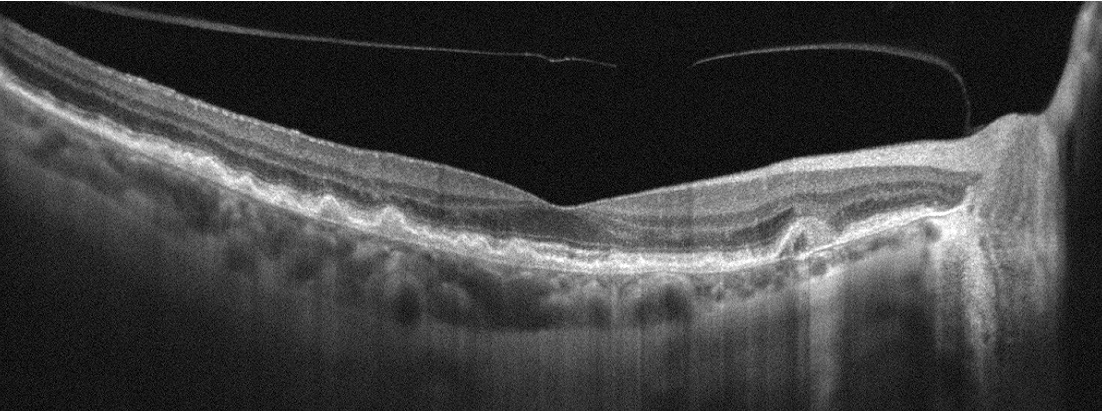

Dx: age-related macular degeneration (AMD).